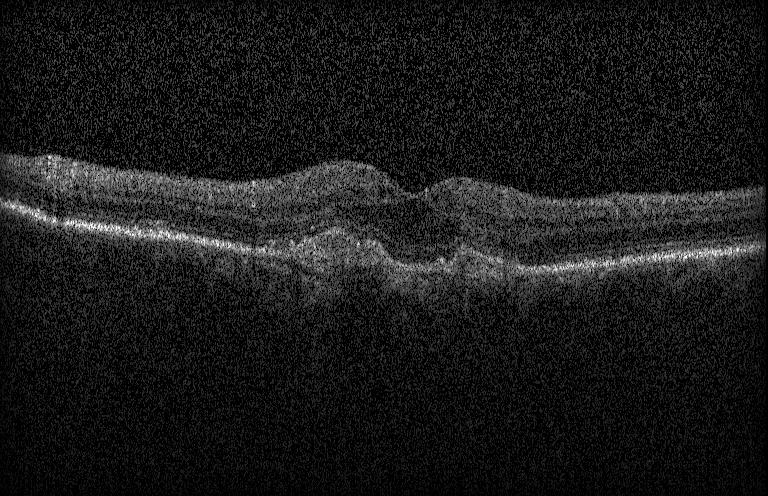
Retinal OCT B-scan.
The scan shows a choroidal neovascular membrane.